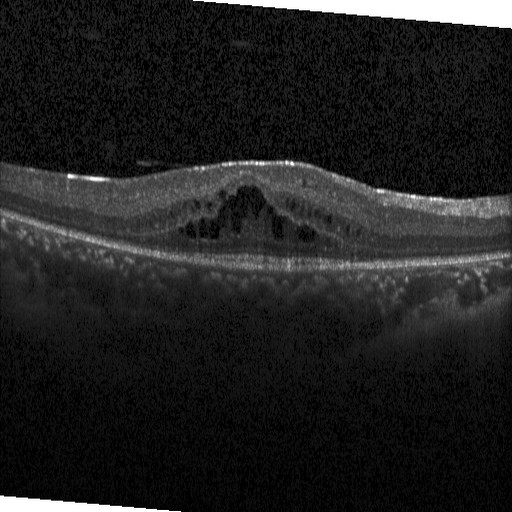

Heidelberg Spectralis; OCT line scan; spectral-domain optical coherence tomography.
The scan shows DME.